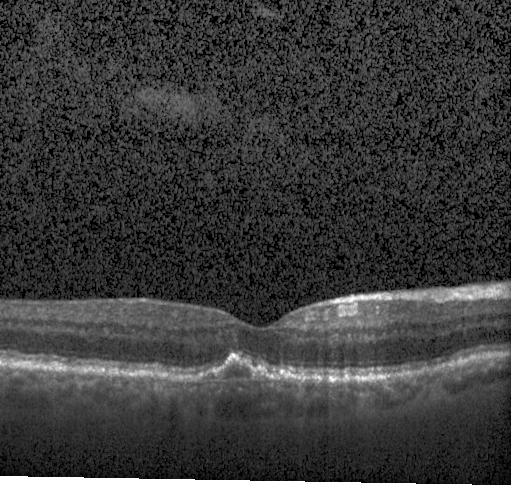 Retinal OCT cross-section showing CNV.